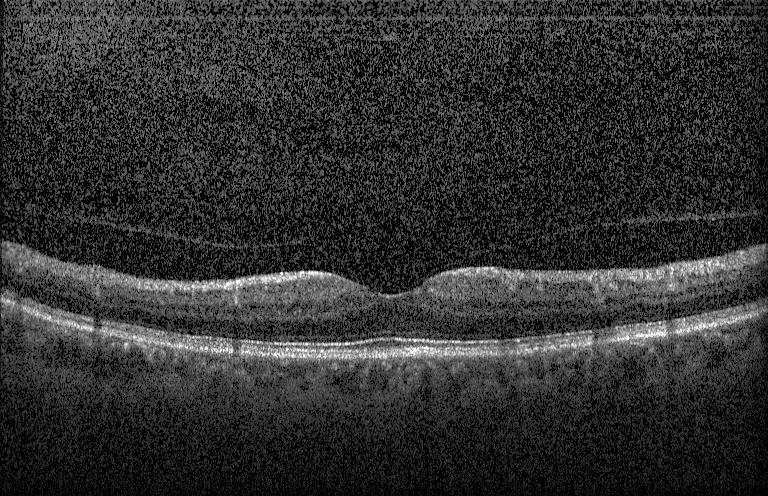 Retinal OCT B-scan. Macular scan. No CNV, DME, or drusen.